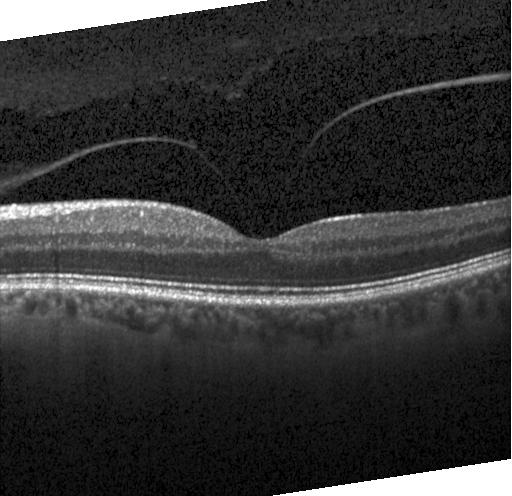

OCT scan showing no choroidal neovascularization, diabetic macular edema, or drusen.